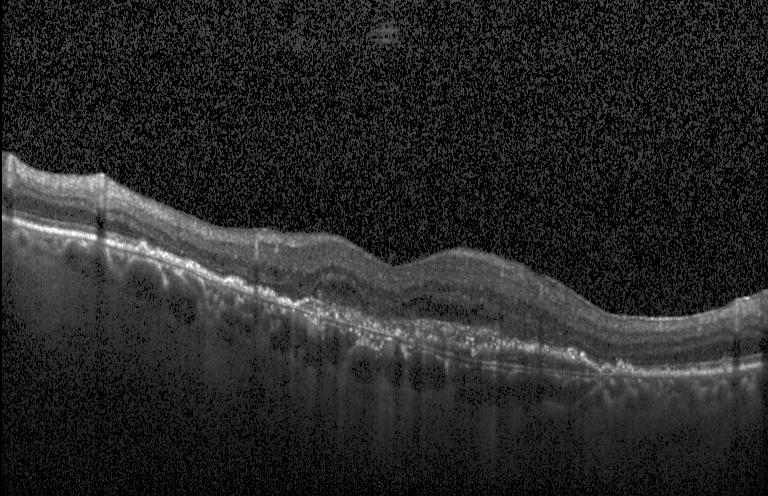
Retinal OCT cross-section, horizontal scan through the fovea, spectral-domain optical coherence tomography.
This B-scan demonstrates a choroidal neovascular membrane.